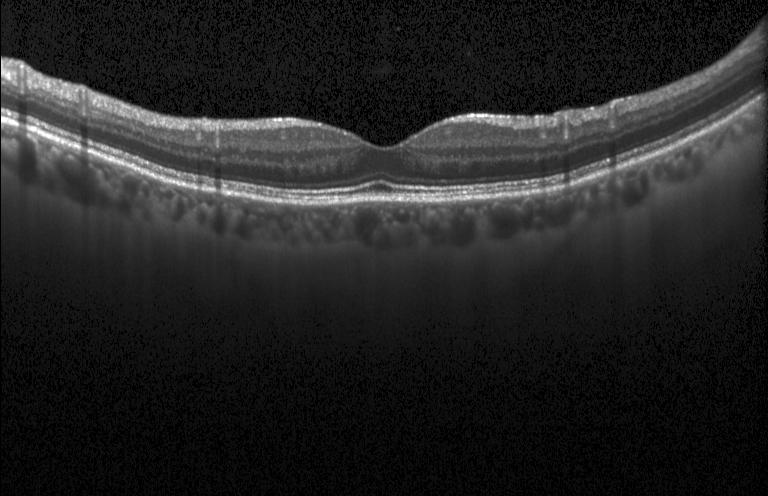 Optical coherence tomography scan · instrument: Heidelberg Spectralis · fovea-centered. This B-scan demonstrates no choroidal neovascularization, diabetic macular edema, or drusen.